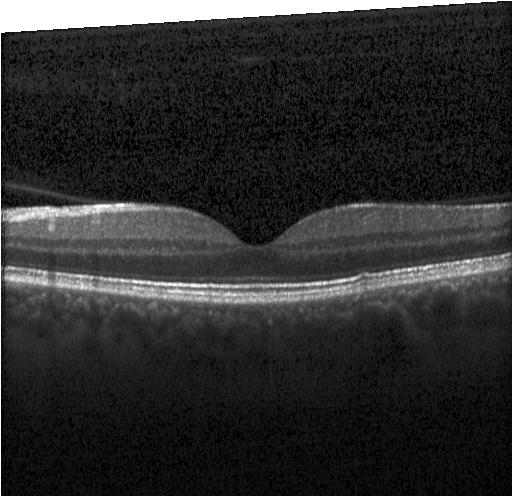 Impression: no choroidal neovascularization, diabetic macular edema, or drusen.